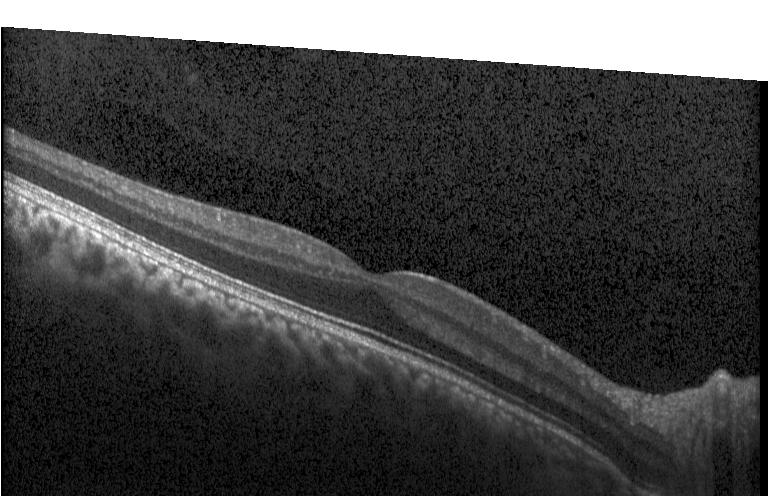 Diagnosis: no choroidal neovascularization, no diabetic macular edema, and no drusen.